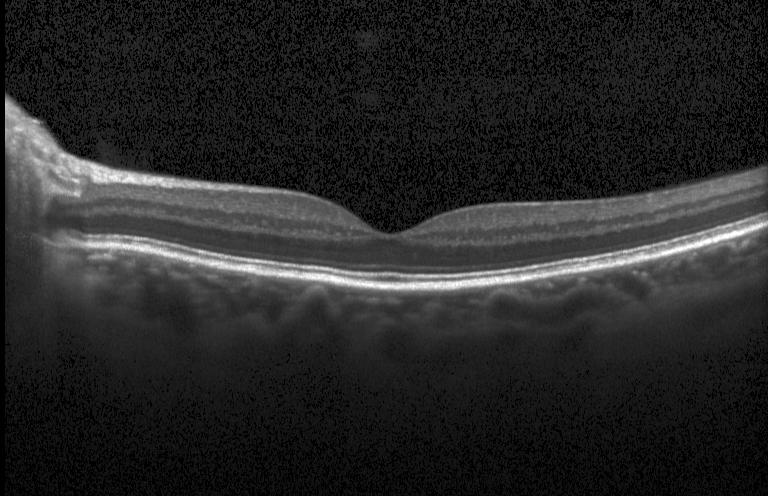

OCT B-scan — Macular OCT: neither choroidal neovascularization, diabetic macular edema, nor drusen.